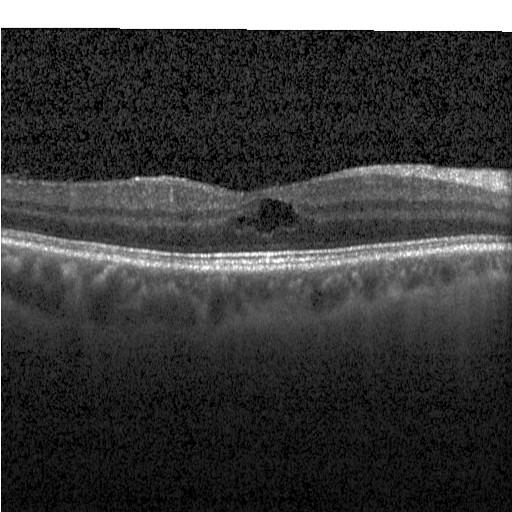 Finding: diabetic macular edema (DME).